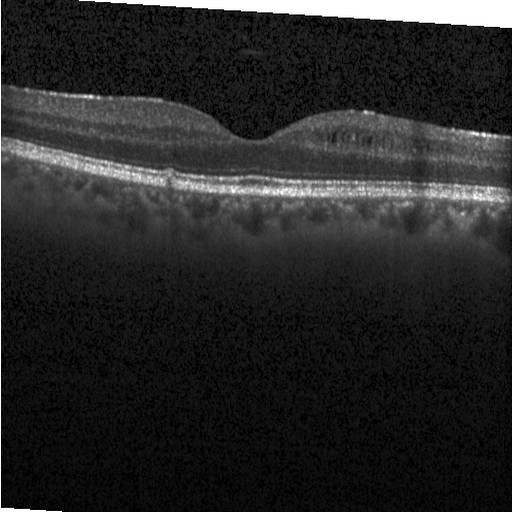
Retinal OCT cross-section showing DME.